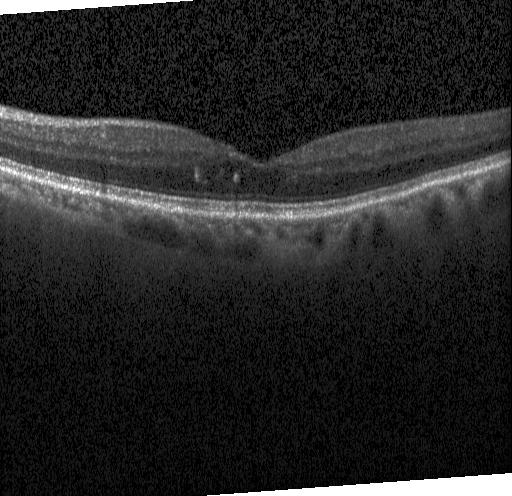 Macular OCT demonstrating no CNV, no DME, and no drusen.